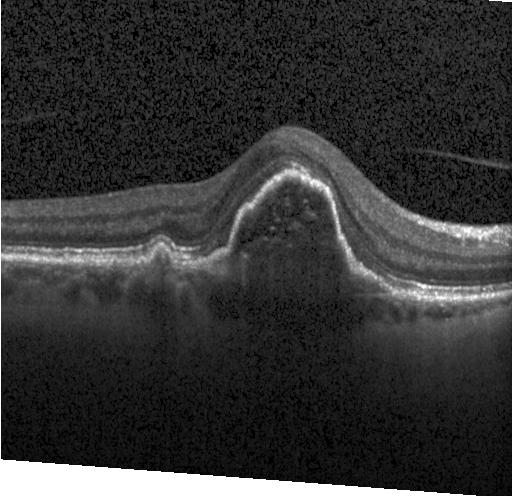 Finding: a choroidal neovascular membrane.